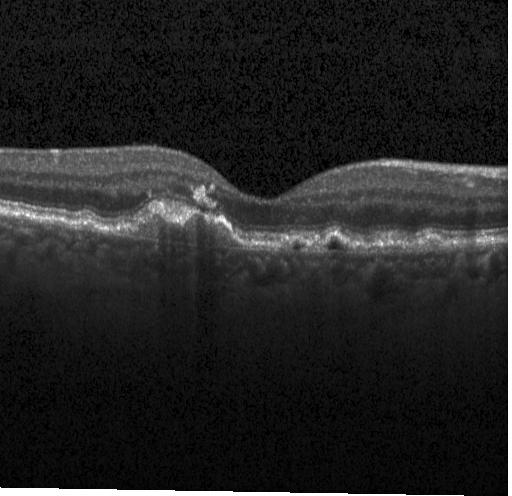

Diagnosis: a choroidal neovascular membrane.